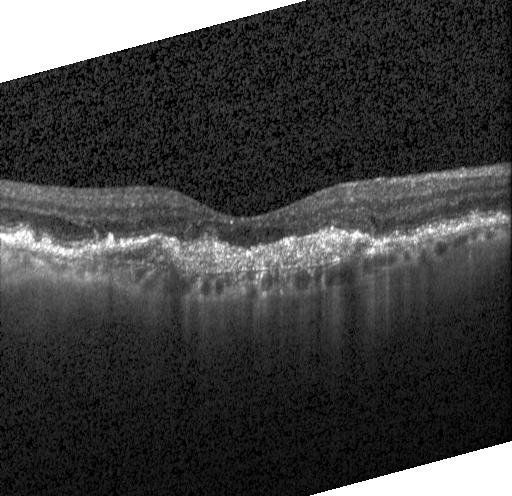

Optical coherence tomography B-scan; spectral-domain optical coherence tomography — Impression: choroidal neovascularization (CNV).